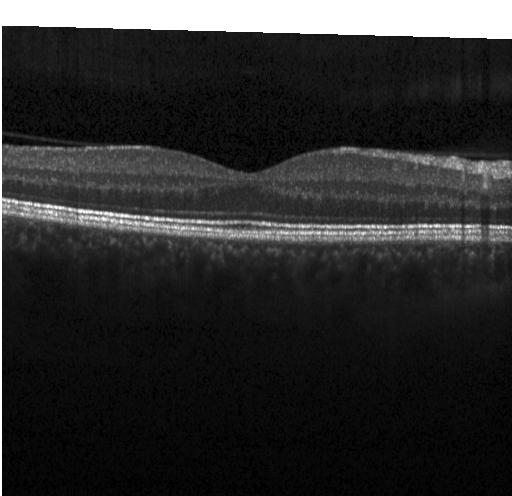

Spectral-domain OCT; through the macula; optical coherence tomography B-scan.
Assessment: no choroidal neovascularization, no diabetic macular edema, and no drusen.